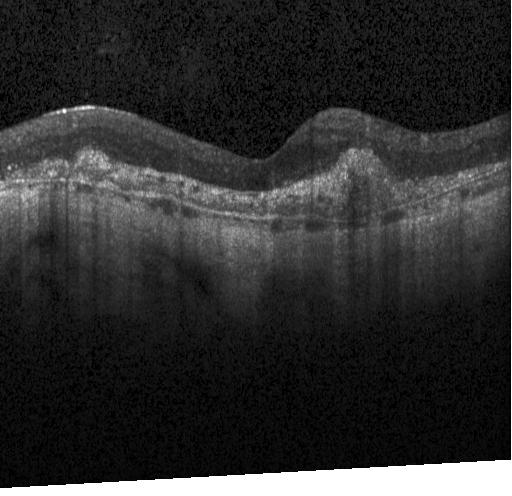

Spectral-domain OCT, retinal OCT cross-section
The scan shows choroidal neovascularization.